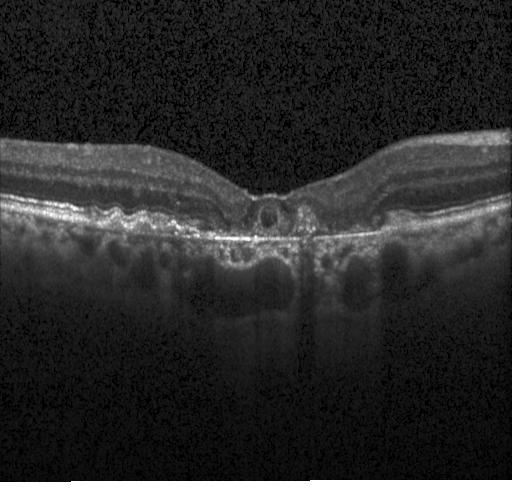 Acquired on a Heidelberg Spectralis; centered on the fovea; SD-OCT; retinal OCT B-scan. Macular OCT: a choroidal neovascular membrane.